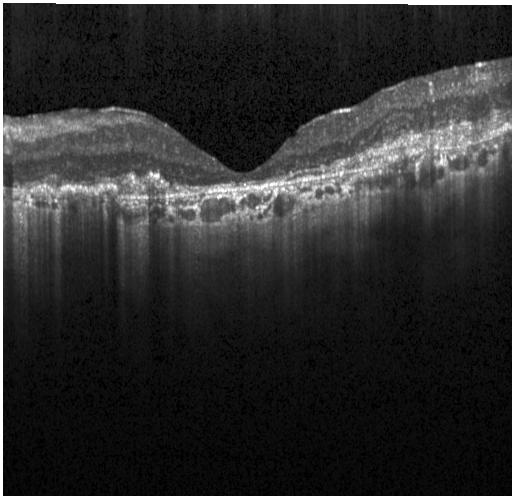 Retinal OCT cross-section; Heidelberg Spectralis; centered on the fovea; SD-OCT. Finding: a choroidal neovascular membrane.